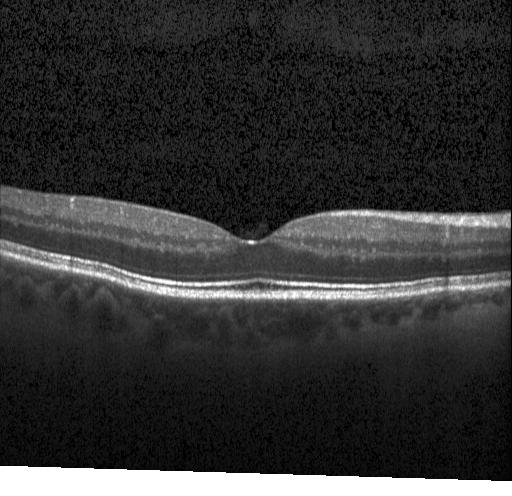

Diagnosis: no choroidal neovascularization, no diabetic macular edema, and no drusen.